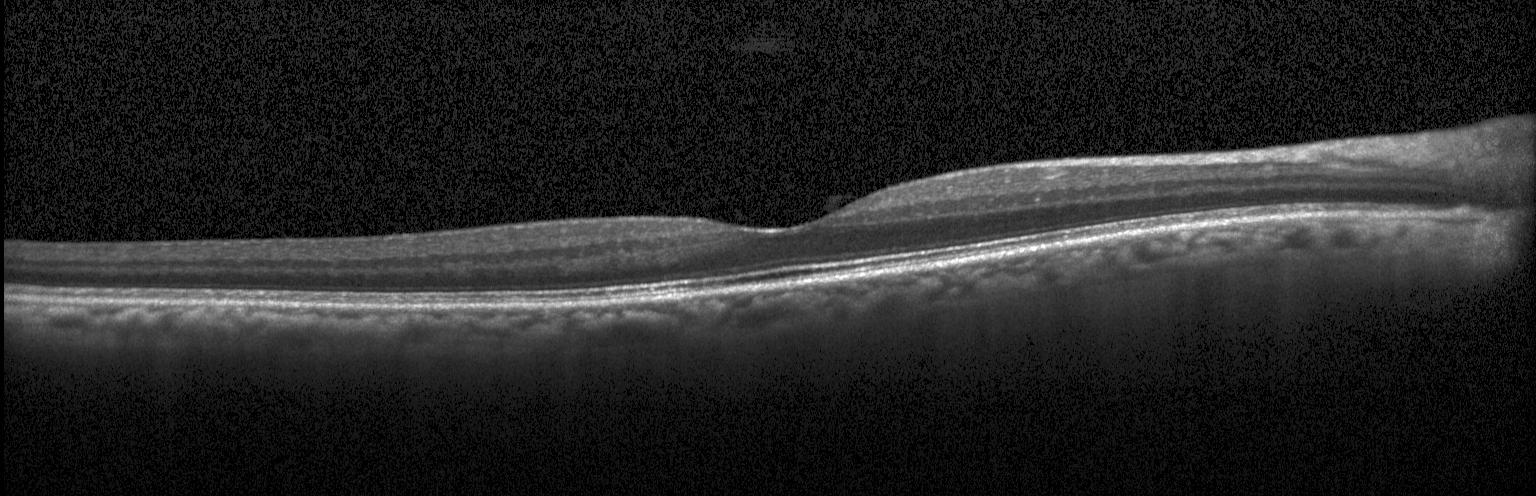
Retinal OCT cross-section. Impression: neither CNV, DME, nor drusen.